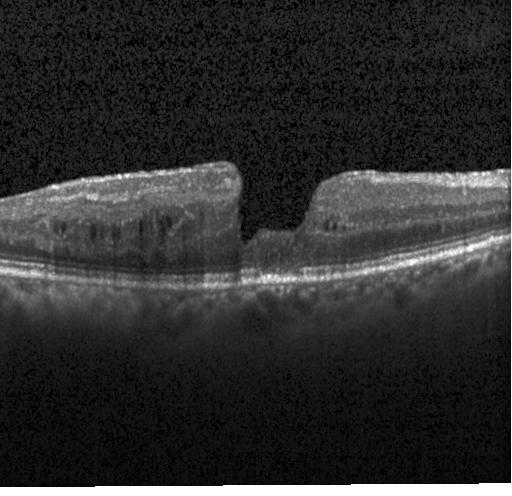
Macular scan · spectral-domain OCT · Heidelberg Spectralis · retinal OCT B-scan. Dx: diabetic macular edema (DME).